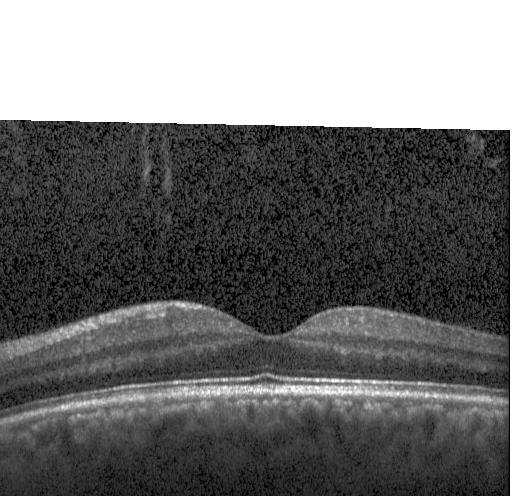
Retinal OCT B-scan.
Impression: no evidence of CNV, DME, or drusen.